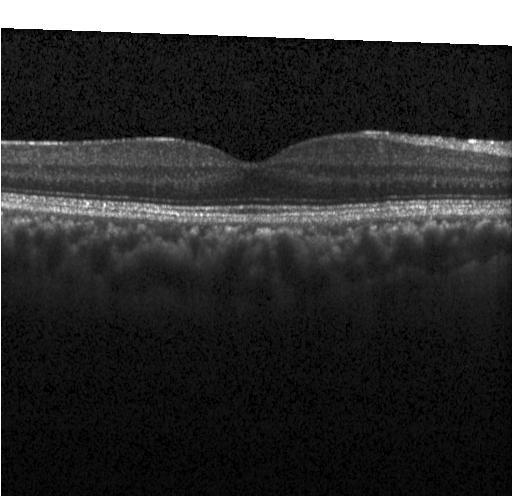

Spectral-domain OCT; through the macula; Heidelberg Spectralis; optical coherence tomography B-scan. No evidence of CNV, DME, or drusen.